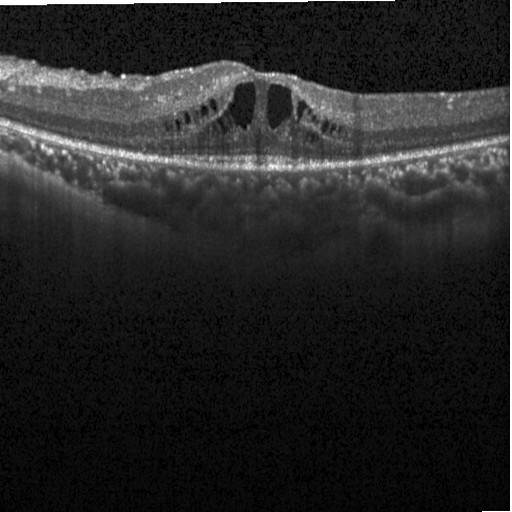

Retinal OCT B-scan · spectral-domain OCT · centered on the fovea
Diagnosis: diabetic macular edema.